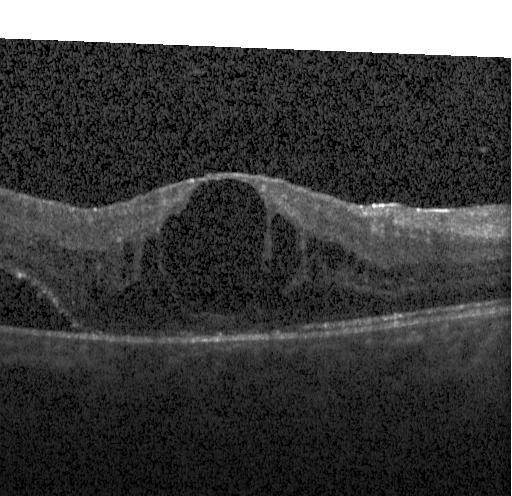
OCT line scan — DME.